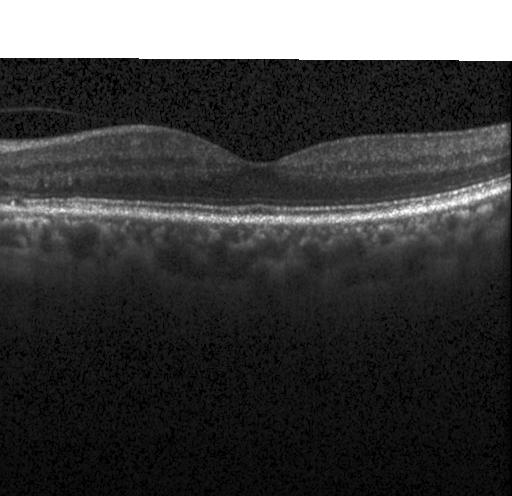
OCT B-scan showing no evidence of CNV, DME, or drusen.